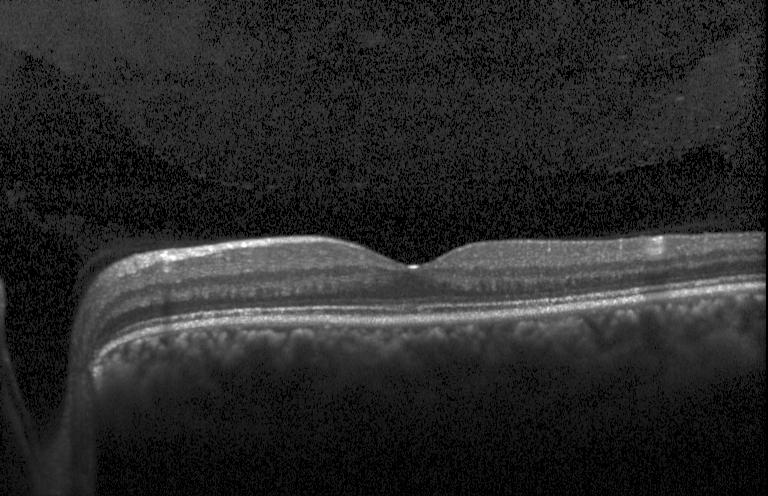
Acquired on a Heidelberg Spectralis. OCT line scan.
Diagnosis: no choroidal neovascularization, no diabetic macular edema, and no drusen.